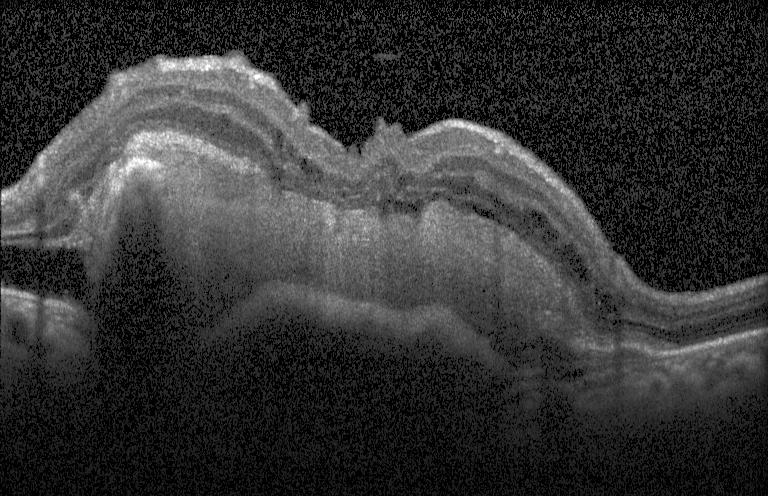

Assessment: a choroidal neovascular membrane.